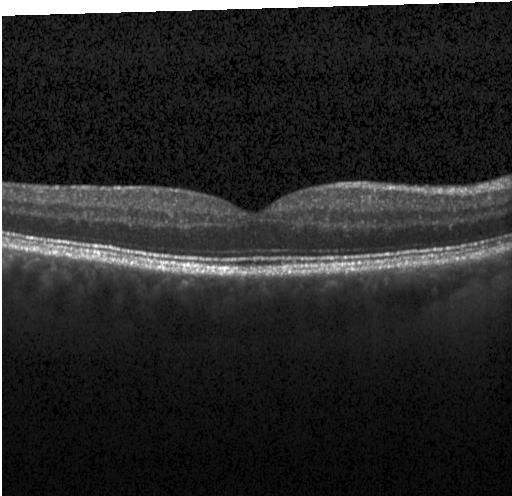 Retinal OCT cross-section, spectral-domain OCT
No evidence of choroidal neovascularization, diabetic macular edema, or drusen.